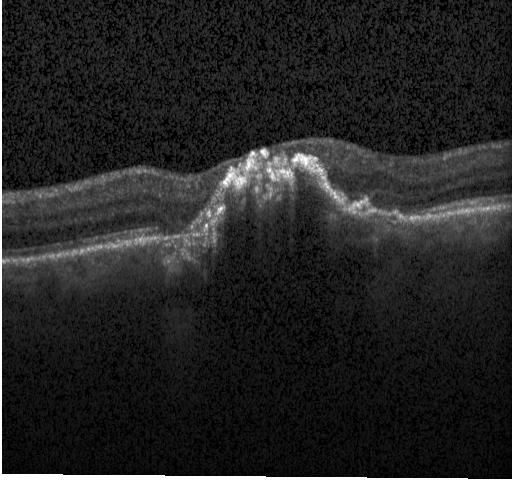

OCT line scan · instrument: Heidelberg Spectralis · centered on the fovea. Diagnosis: a choroidal neovascular membrane.